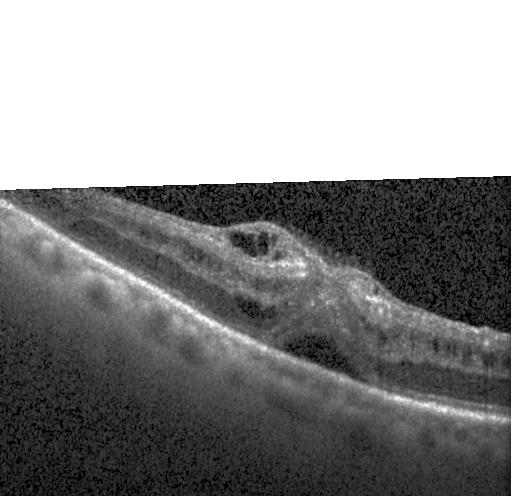

OCT B-scan. Macular OCT: diabetic macular edema.